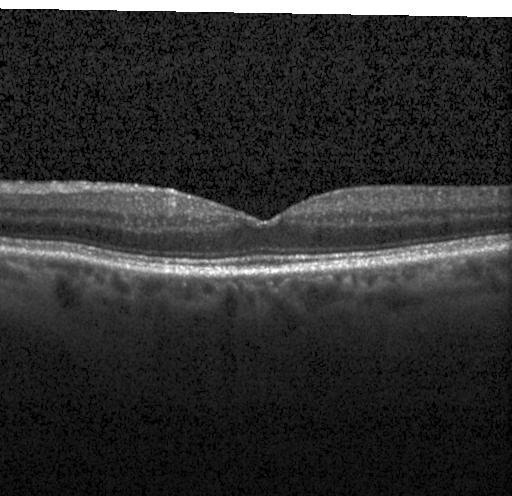 Impression: no evidence of CNV, DME, or drusen.